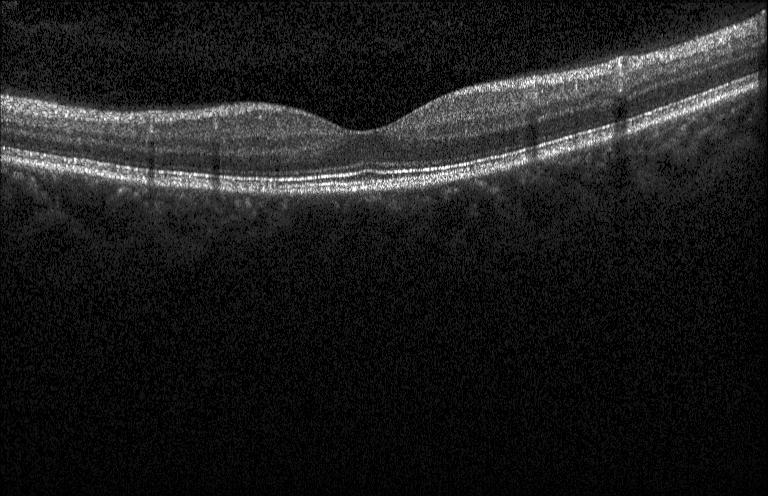
Diagnosis: neither CNV, DME, nor drusen.